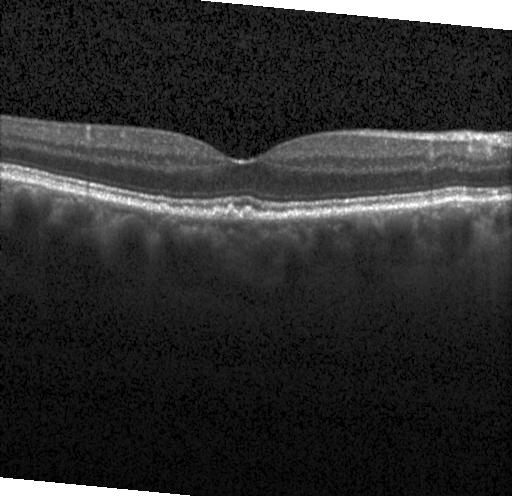
OCT scan showing multiple drusen.